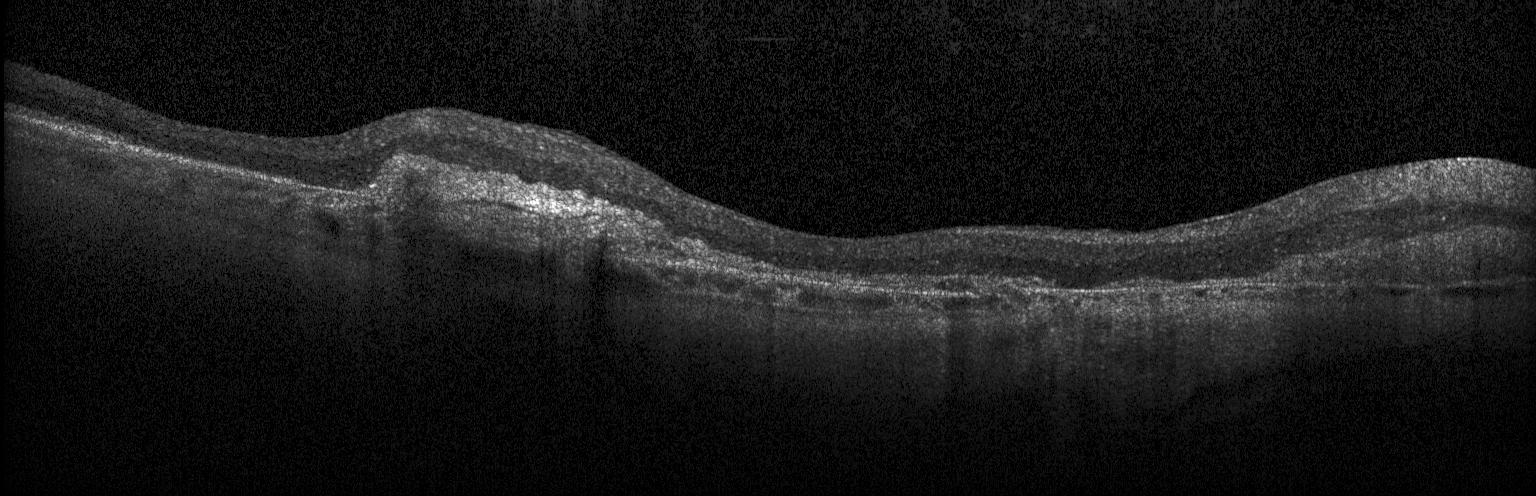

OCT B-scan
This B-scan demonstrates CNV.